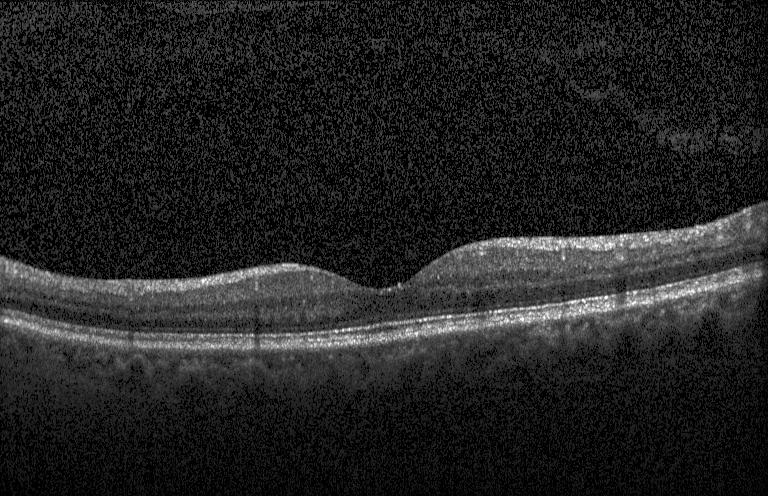

Retinal OCT cross-section — The scan shows no choroidal neovascularization, no diabetic macular edema, and no drusen.